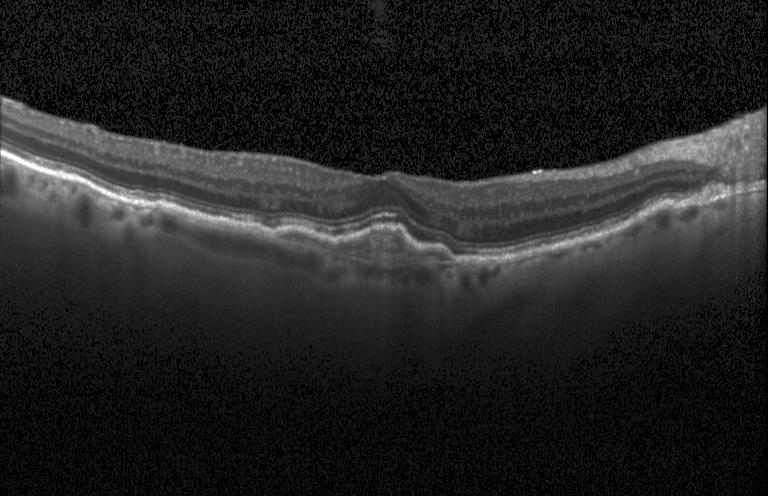
Impression: a choroidal neovascular membrane.